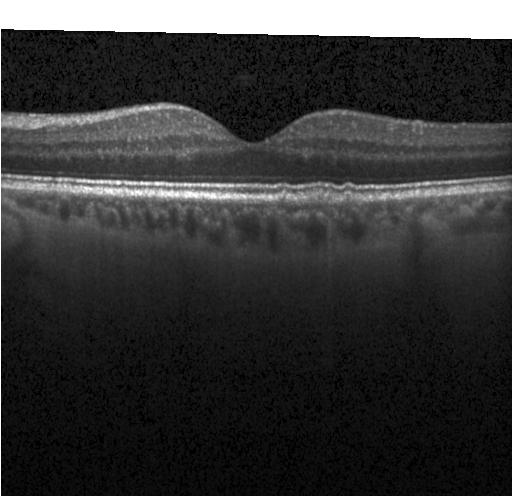

Impression: drusen.